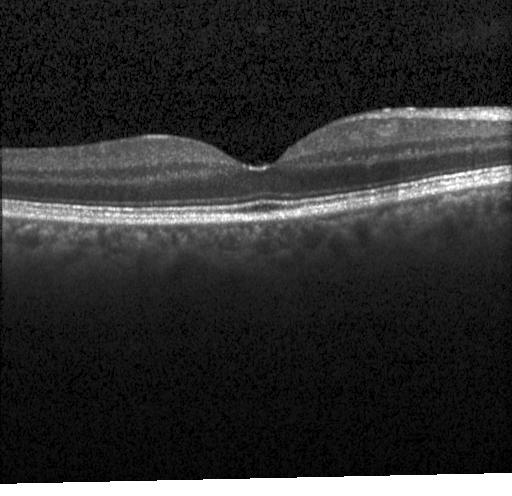 Optical coherence tomography B-scan, Heidelberg Spectralis, horizontal scan through the fovea.
Assessment: no choroidal neovascularization, diabetic macular edema, or drusen.